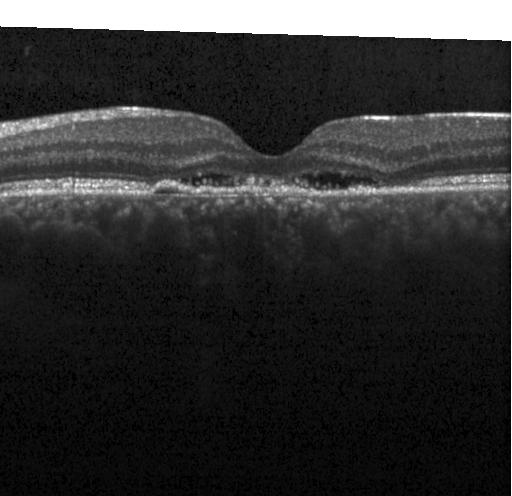

Horizontal scan through the fovea. Spectral-domain optical coherence tomography. Acquired on a Heidelberg Spectralis. Retinal OCT cross-section.
Finding: choroidal neovascularization (CNV).